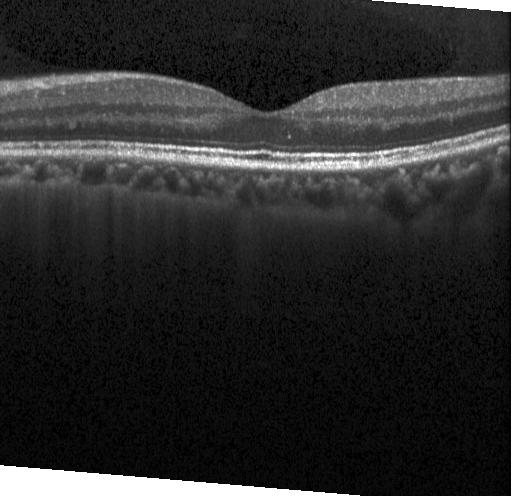

Spectral-domain OCT; retinal OCT B-scan
Finding: no evidence of choroidal neovascularization, diabetic macular edema, or drusen.